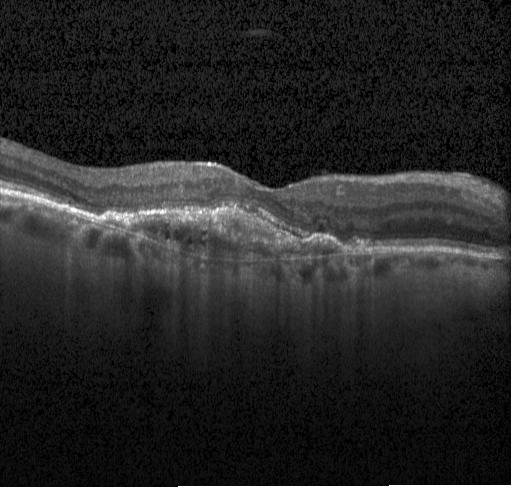

OCT B-scan showing CNV.